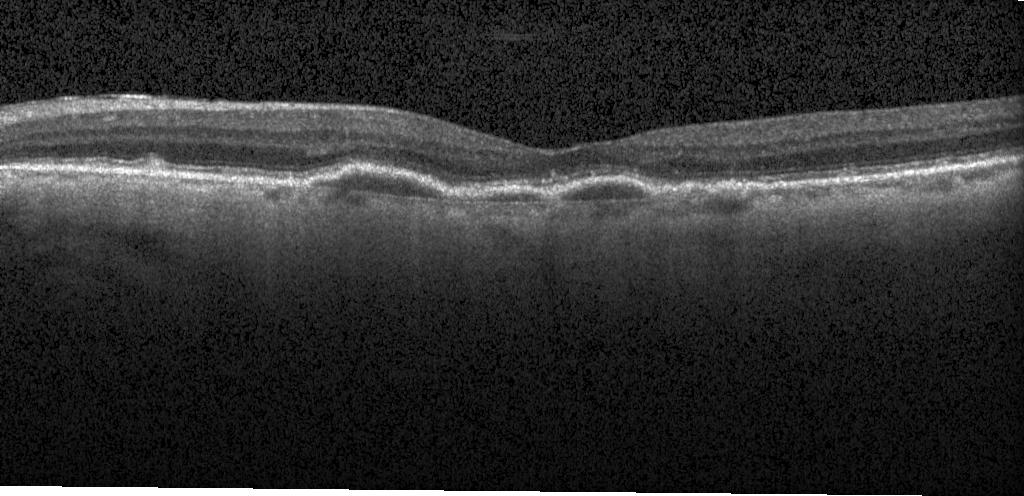
OCT B-scan — Macular OCT: choroidal neovascularization (CNV).